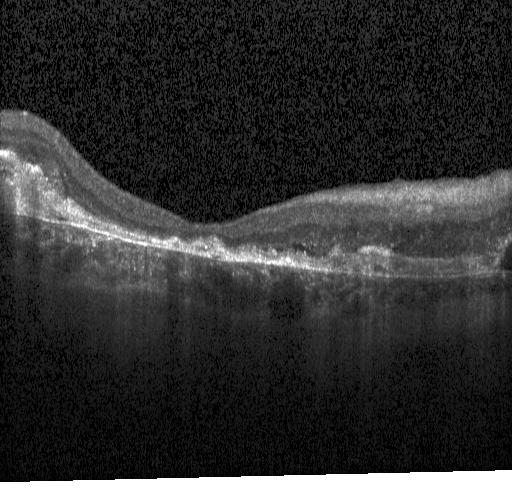
Diagnosis: a choroidal neovascular membrane.